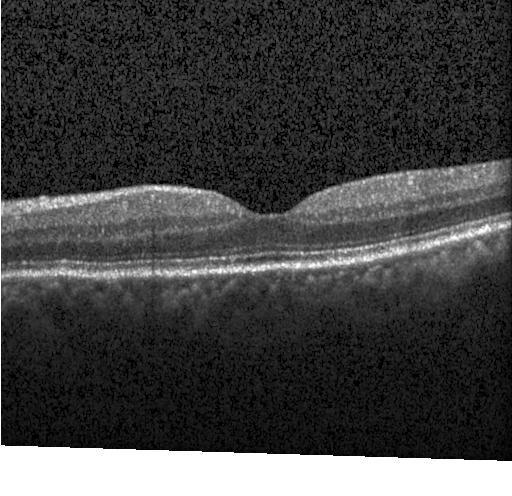

Optical coherence tomography B-scan
Finding: no CNV, no DME, and no drusen.